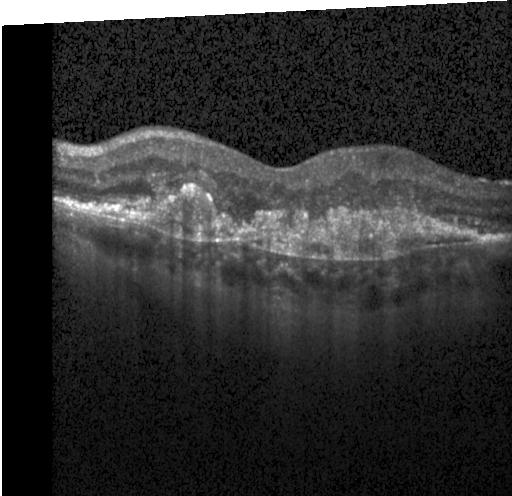
Heidelberg Spectralis, spectral-domain OCT, OCT B-scan, fovea-centered
This B-scan demonstrates a choroidal neovascular membrane.